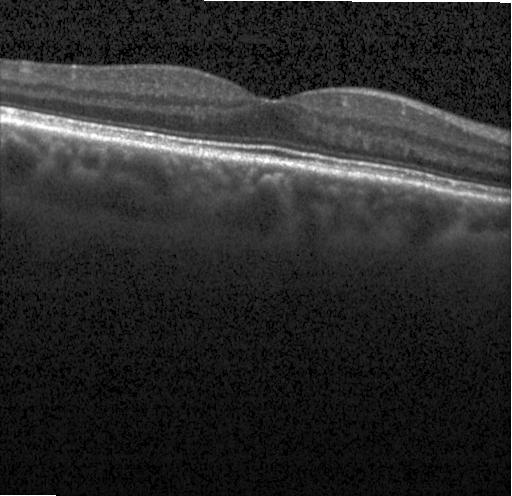

Finding: no choroidal neovascularization, no diabetic macular edema, and no drusen.